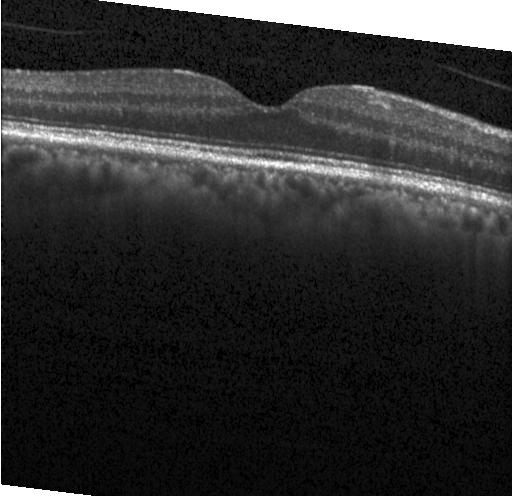 Heidelberg Spectralis. Spectral-domain OCT. OCT line scan. Horizontal scan through the fovea — Impression: no choroidal neovascularization, no diabetic macular edema, and no drusen.